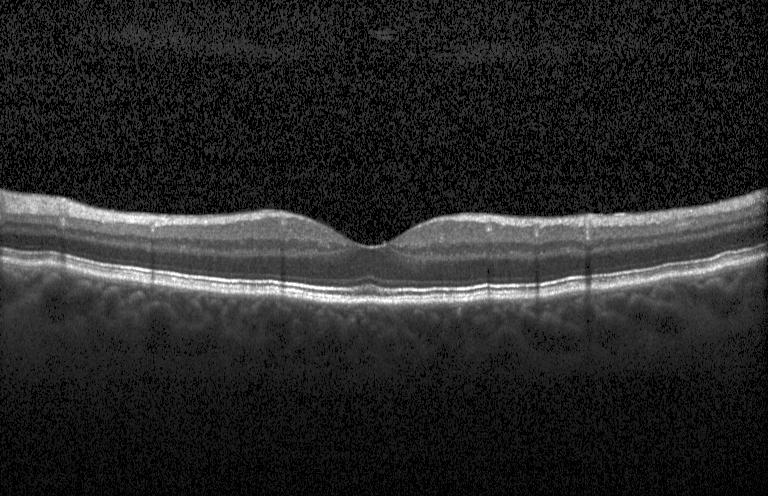

Instrument: Heidelberg Spectralis; retinal OCT cross-section
This B-scan demonstrates neither choroidal neovascularization, diabetic macular edema, nor drusen.